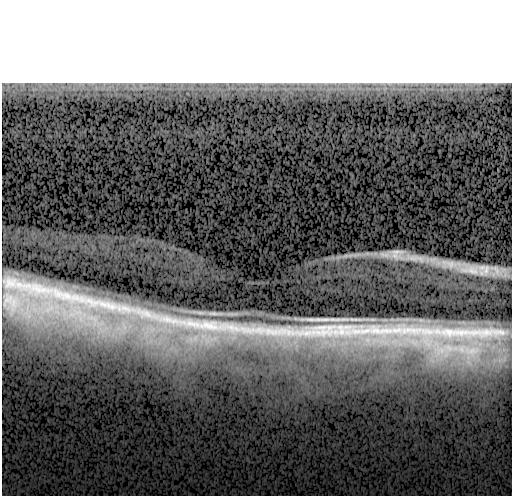

OCT B-scan showing no choroidal neovascularization, diabetic macular edema, or drusen.